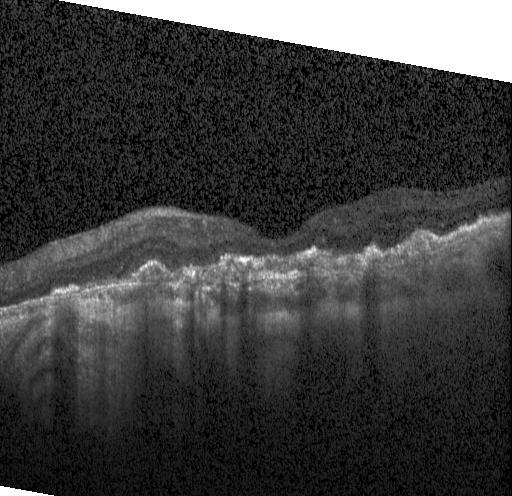 Retinal OCT cross-section showing choroidal neovascularization.